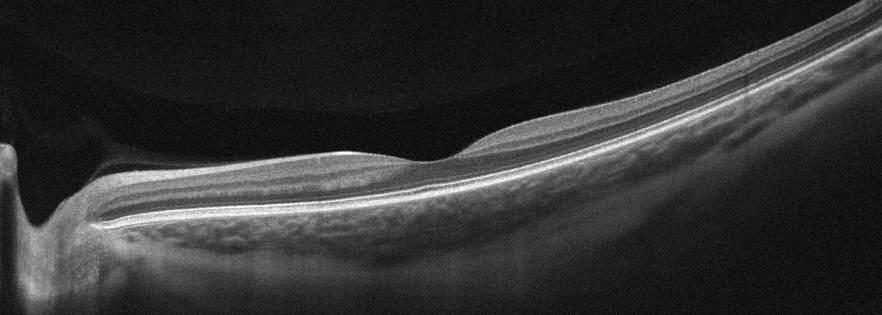 Optical coherence tomography scan; through the macula; OS.
Impression: absence of AMD, DME, ERM, RAO, RVO, and vitreomacular interface disease.